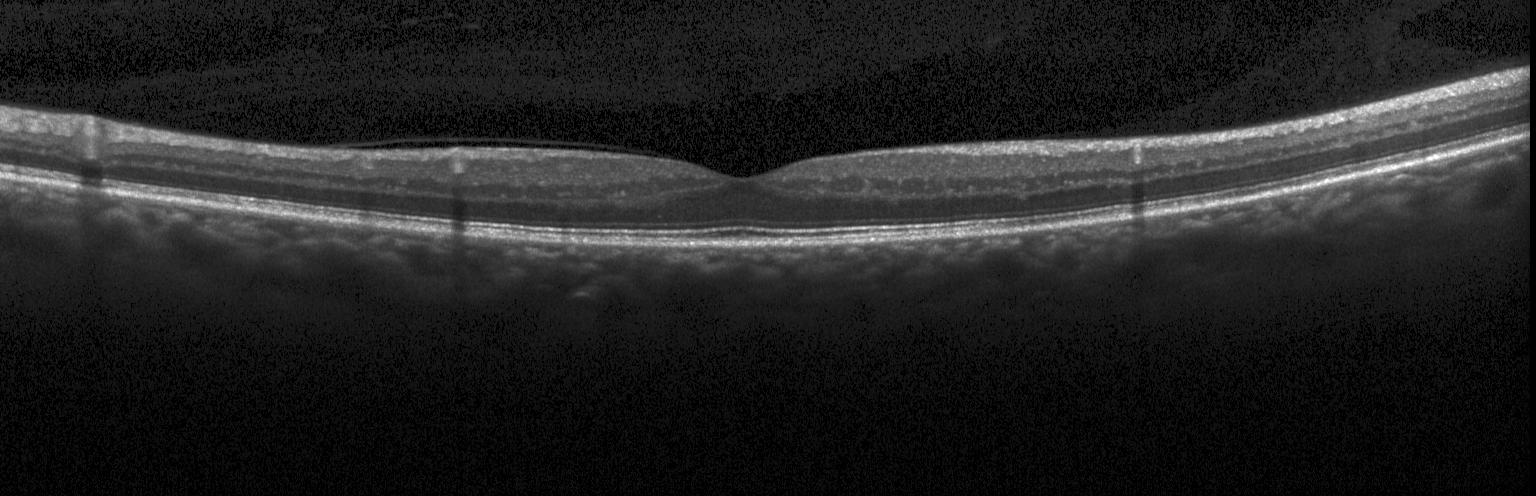
OCT B-scan, spectral-domain optical coherence tomography
This B-scan demonstrates no evidence of CNV, DME, or drusen.